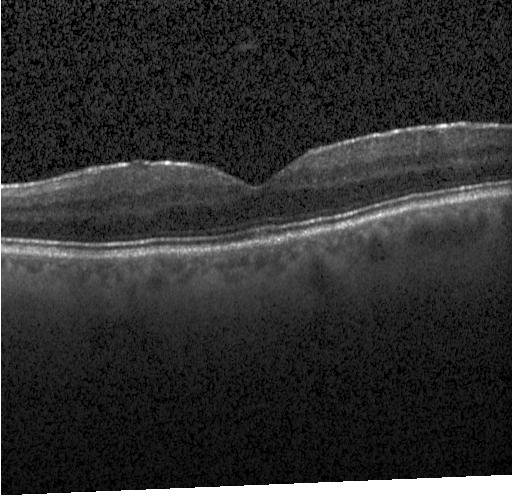

Heidelberg Spectralis OCT system, spectral-domain OCT, through the macula, optical coherence tomography scan. Finding: no CNV, no DME, and no drusen.